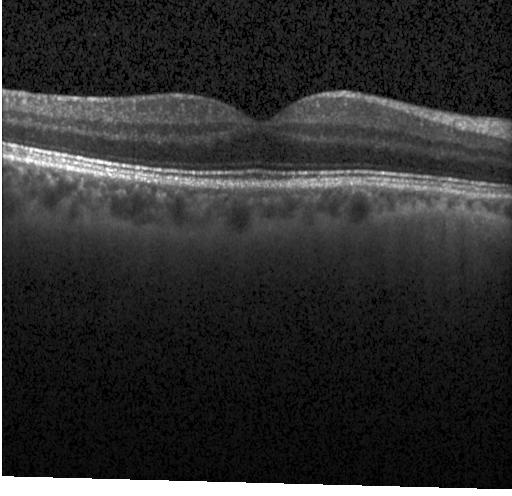

OCT line scan; spectral-domain optical coherence tomography; through the macula — No choroidal neovascularization, diabetic macular edema, or drusen.